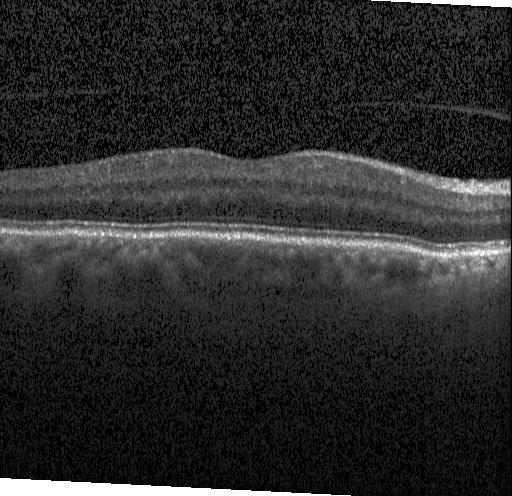

Macular OCT demonstrating neither choroidal neovascularization, diabetic macular edema, nor drusen.